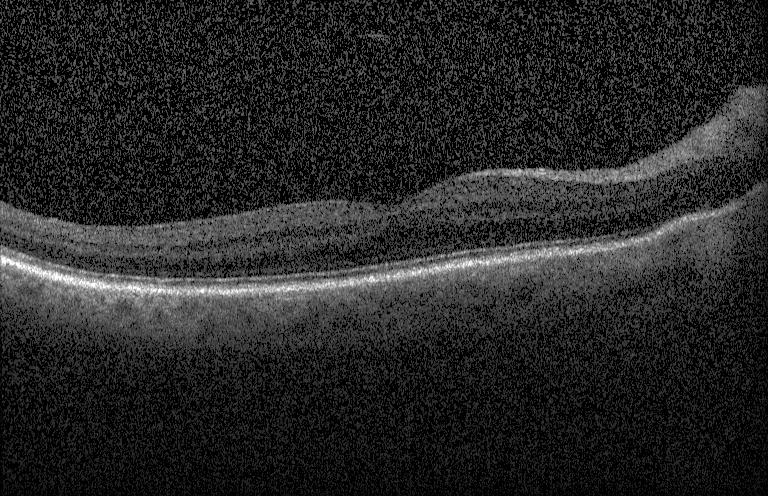 Dx: no CNV, no DME, and no drusen.